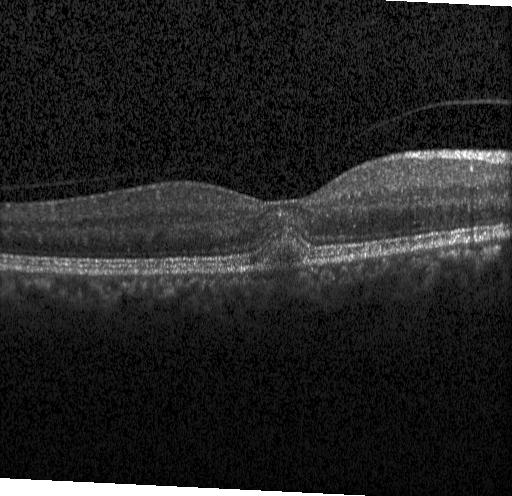

OCT finding: choroidal neovascularization.